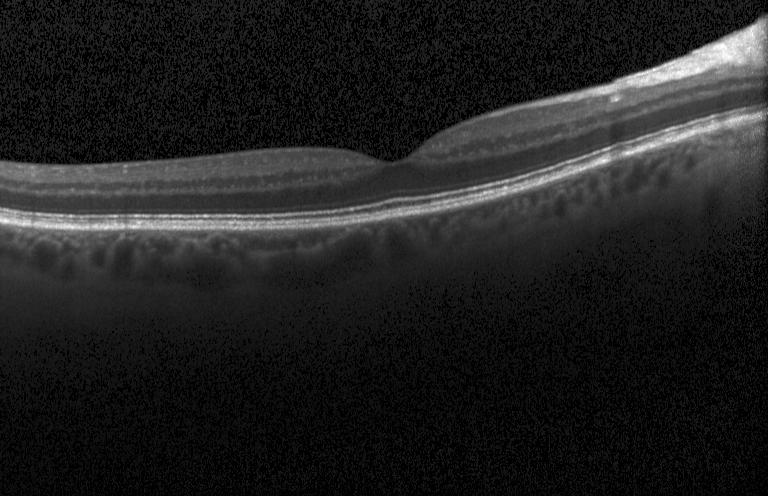 Heidelberg Spectralis · OCT B-scan · spectral-domain OCT — This B-scan demonstrates no evidence of choroidal neovascularization, diabetic macular edema, or drusen.